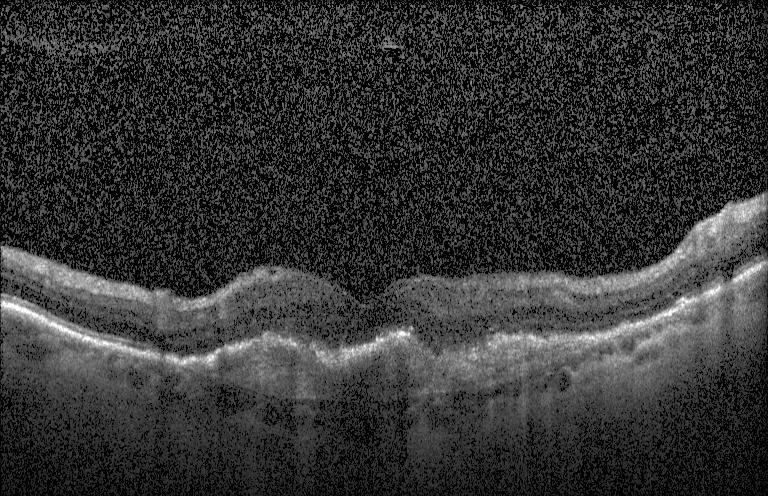
OCT B-scan. Choroidal neovascularization.